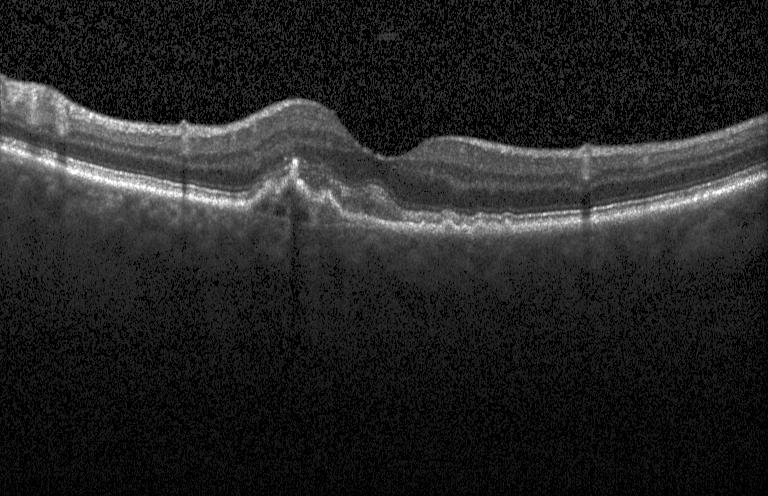 Macular OCT: CNV.